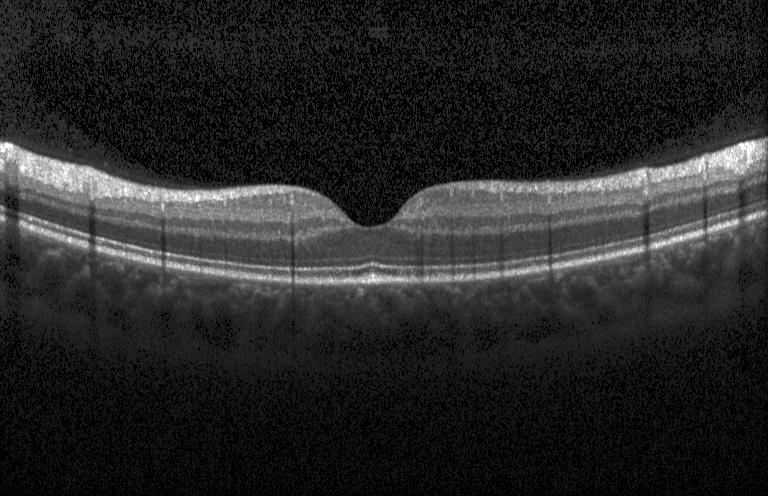

Instrument: Heidelberg Spectralis. Horizontal scan through the fovea. Retinal OCT B-scan
Diagnosis: no CNV, no DME, and no drusen.